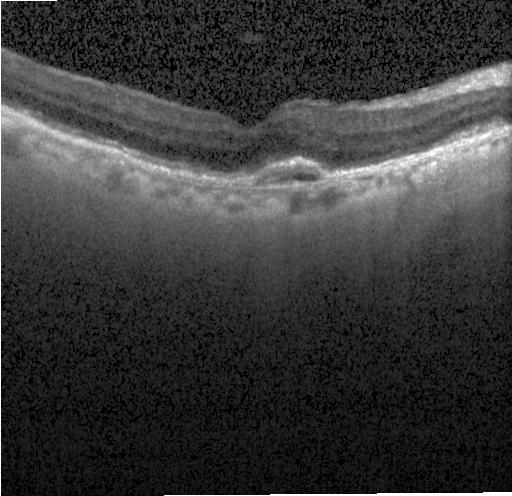
Retinal OCT B-scan · horizontal scan through the fovea · spectral-domain OCT · Heidelberg Spectralis. This B-scan demonstrates a choroidal neovascular membrane.